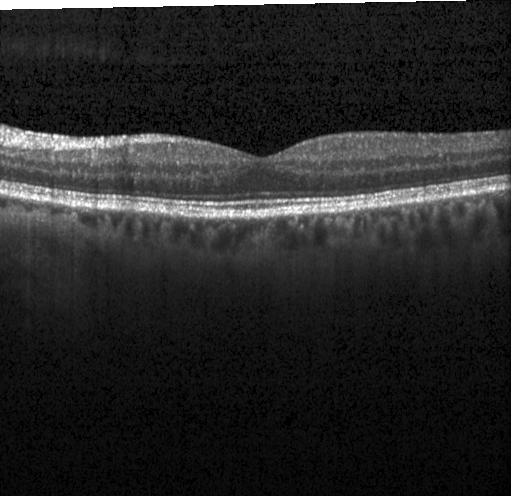
OCT B-scan. Spectral-domain optical coherence tomography. Impression: no evidence of CNV, DME, or drusen.